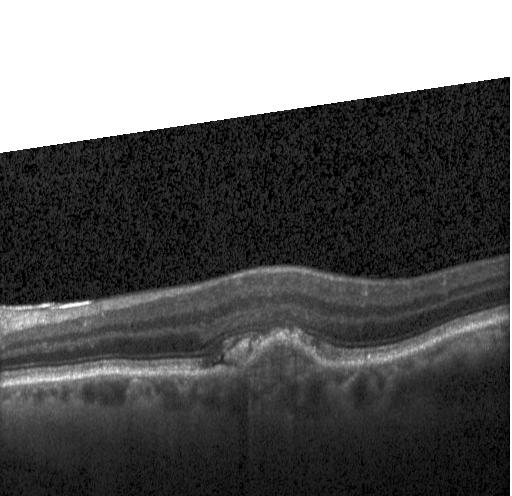
Dx: a choroidal neovascular membrane.